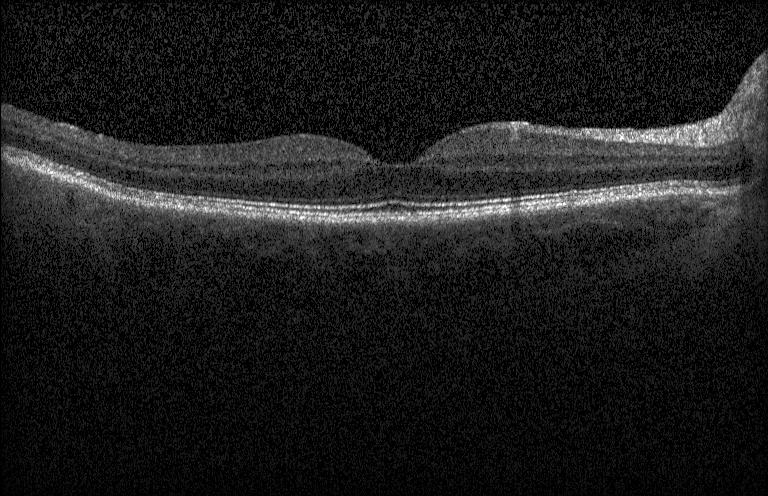
OCT B-scan showing no CNV, no DME, and no drusen.